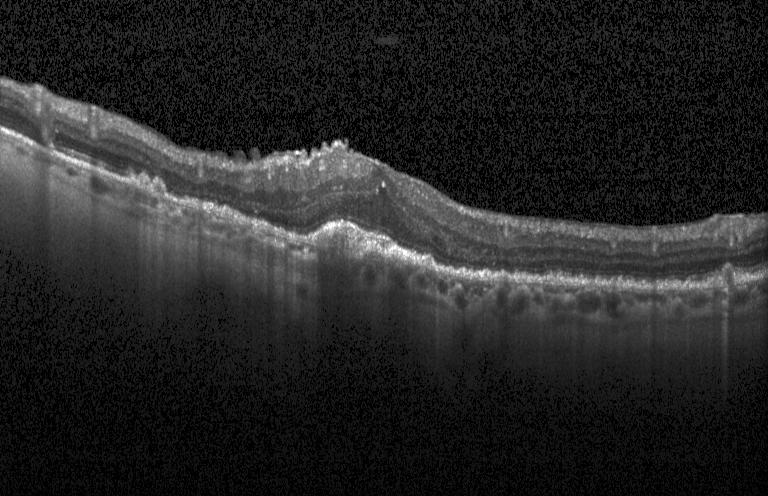 Dx: a choroidal neovascular membrane.